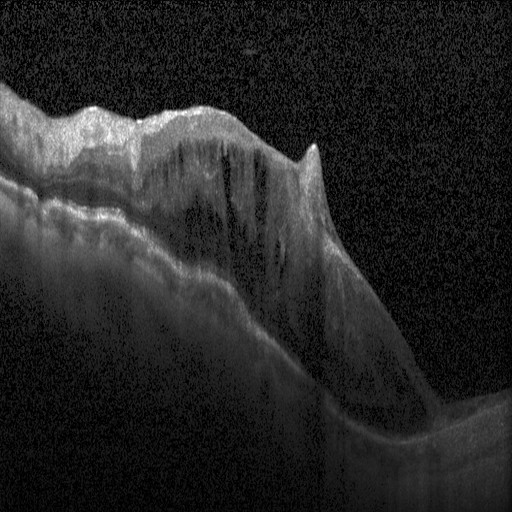 OCT B-scan, centered on the fovea.
Diagnosis: DME.